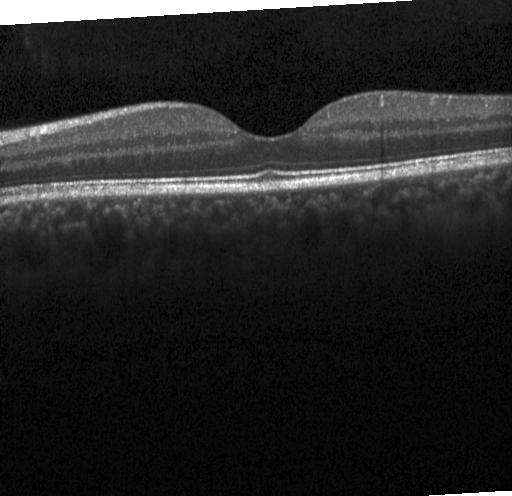
Dx: no evidence of choroidal neovascularization, diabetic macular edema, or drusen.